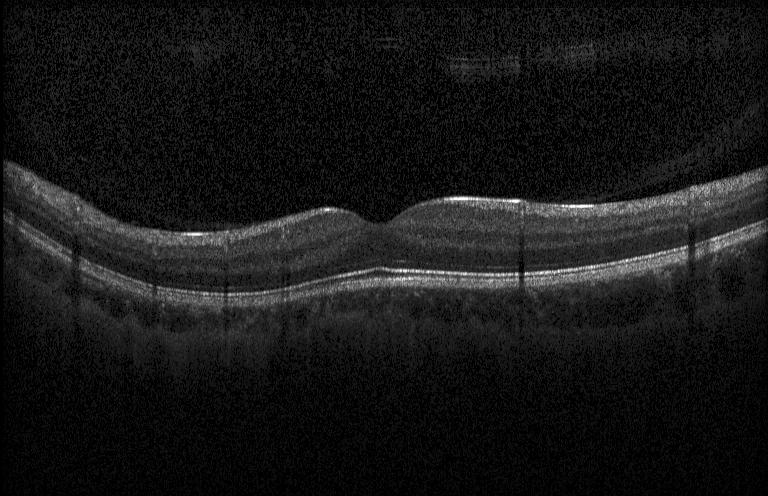 Dx: no choroidal neovascularization, no diabetic macular edema, and no drusen.